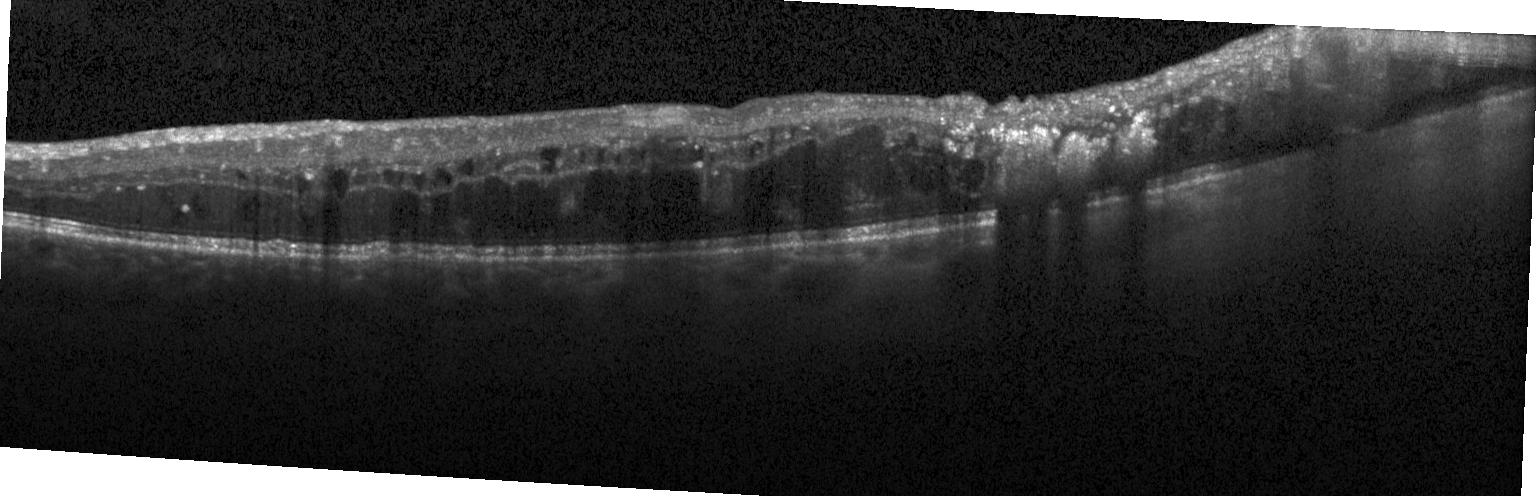
Acquired on a Heidelberg Spectralis · through the macula · SD-OCT · OCT B-scan.
Assessment: DME.